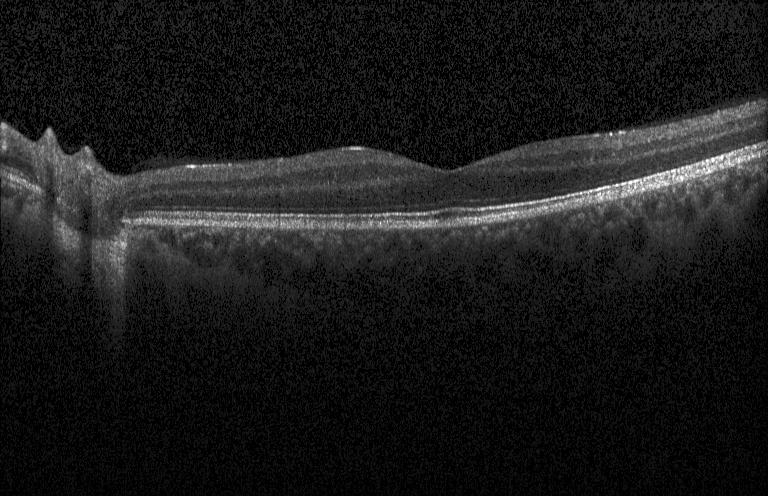
Optical coherence tomography B-scan · Heidelberg Spectralis · horizontal scan through the fovea.
Impression: no evidence of choroidal neovascularization, diabetic macular edema, or drusen.